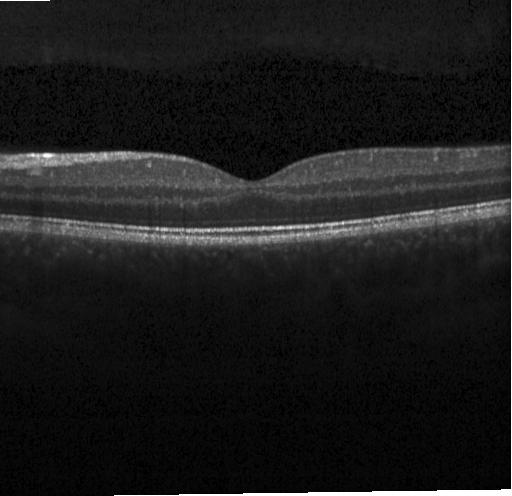
No evidence of choroidal neovascularization, diabetic macular edema, or drusen.